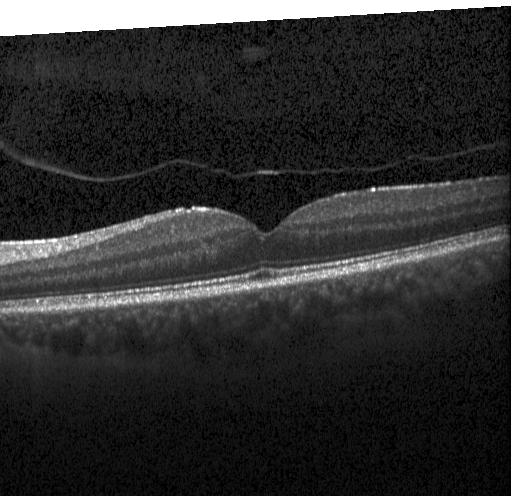

Heidelberg Spectralis OCT system · OCT line scan
Assessment: neither choroidal neovascularization, diabetic macular edema, nor drusen.